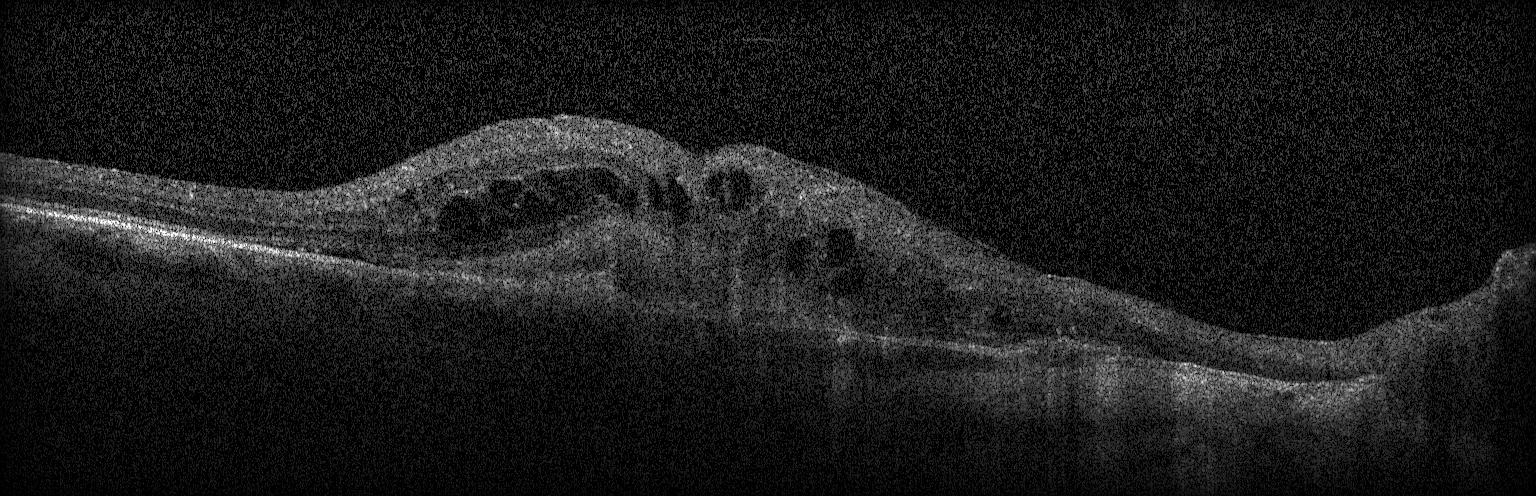

Fovea-centered; OCT line scan — Impression: a choroidal neovascular membrane.